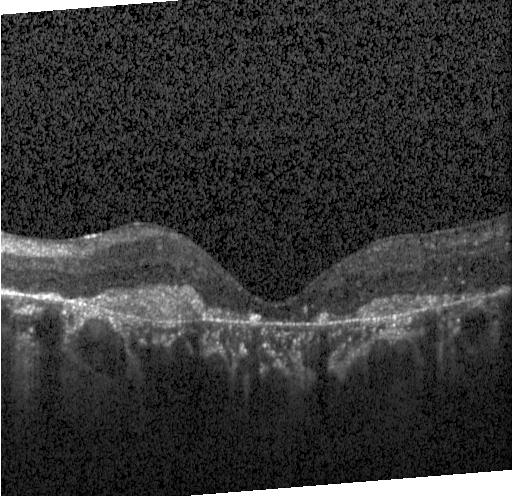 Retinal OCT B-scan, Heidelberg Spectralis OCT system. Macular OCT: CNV.